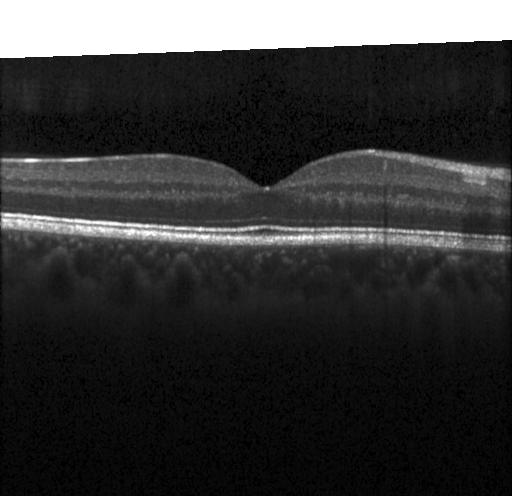

Spectral-domain optical coherence tomography, retinal OCT B-scan — Impression: no evidence of choroidal neovascularization, diabetic macular edema, or drusen.